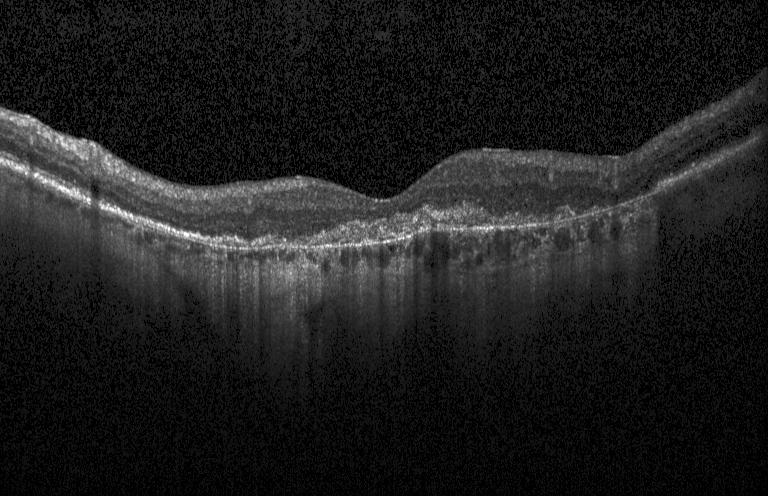

This B-scan demonstrates a choroidal neovascular membrane.